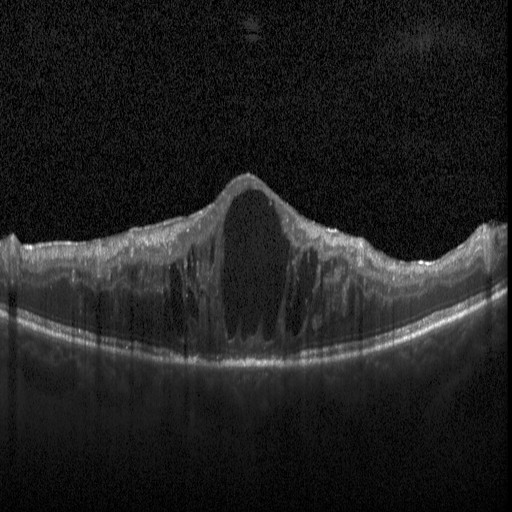

Horizontal scan through the fovea. Instrument: Heidelberg Spectralis. OCT line scan. Dx: DME.